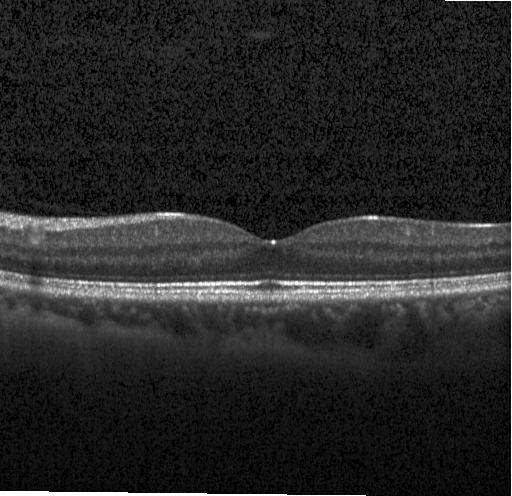

Retinal OCT cross-section. OCT finding: neither choroidal neovascularization, diabetic macular edema, nor drusen.